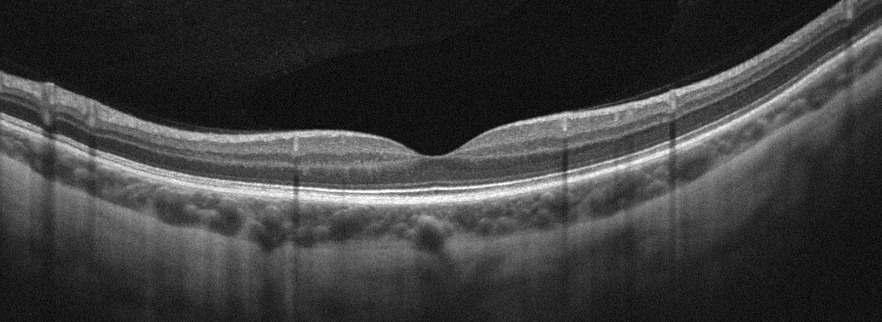

Optical coherence tomography B-scan — This B-scan demonstrates no AMD, DME, ERM, RAO, RVO, or VID.